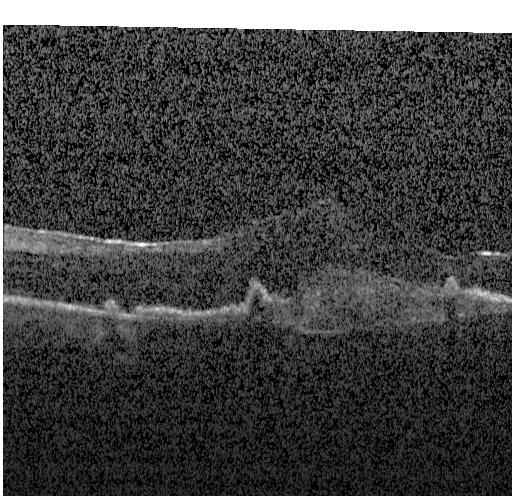 OCT line scan, fovea-centered, spectral-domain OCT. Diagnosis: a choroidal neovascular membrane.